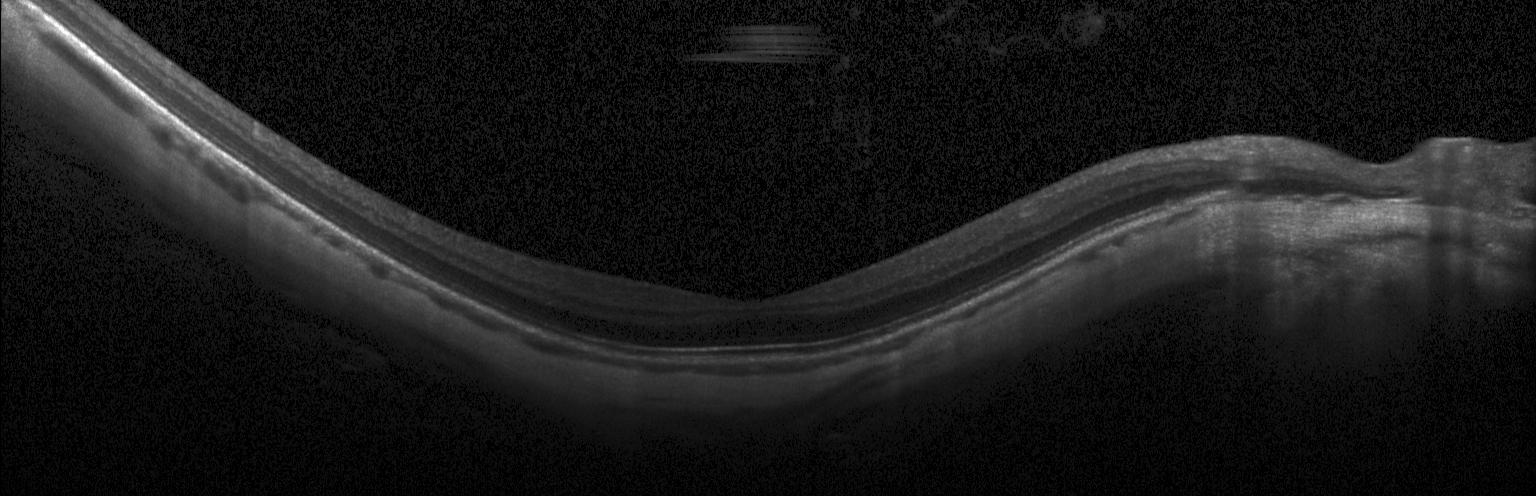

OCT B-scan showing no choroidal neovascularization, diabetic macular edema, or drusen.